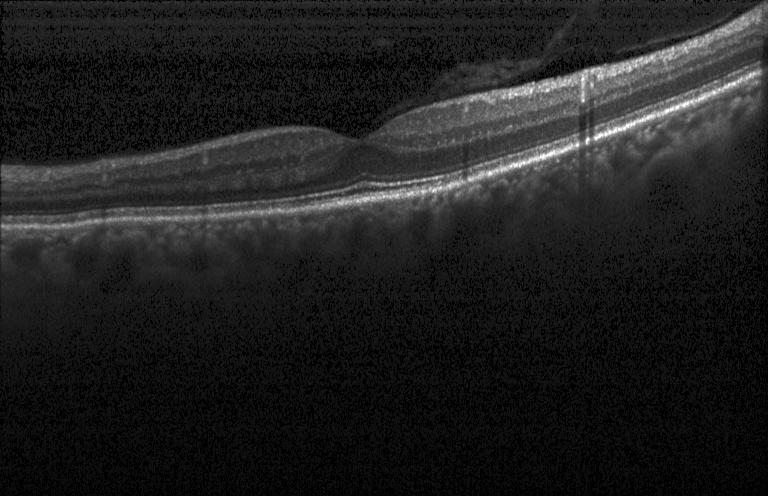 OCT finding: no choroidal neovascularization, diabetic macular edema, or drusen.